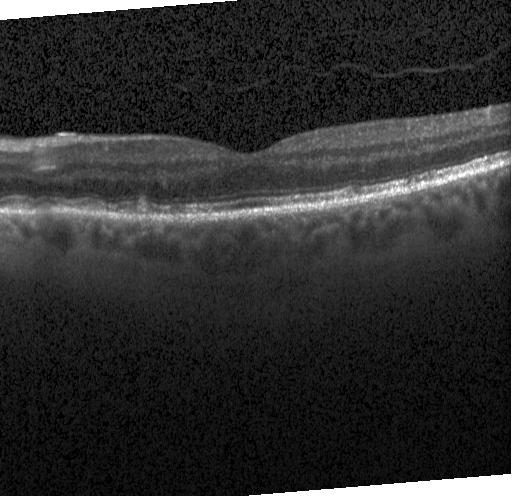
OCT finding: sub-RPE drusenoid deposits.